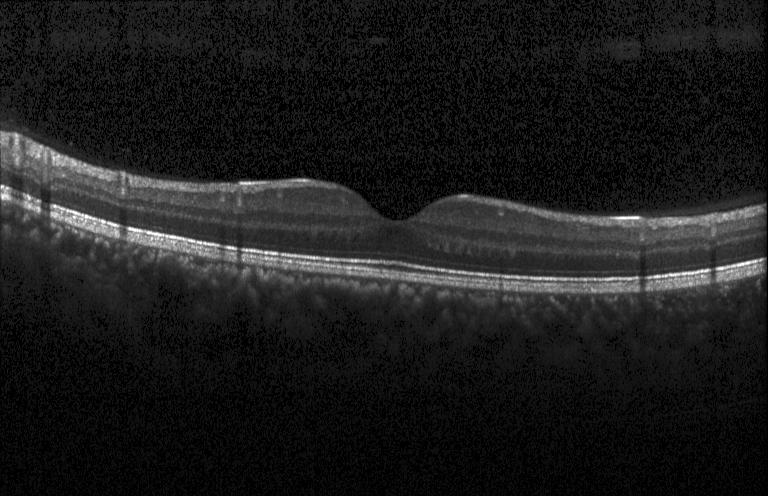
Spectral-domain optical coherence tomography. Retinal OCT cross-section
No CNV, no DME, and no drusen.